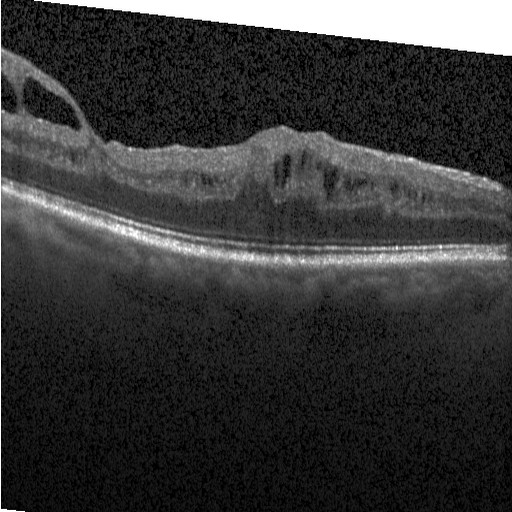 Macular OCT: DME.